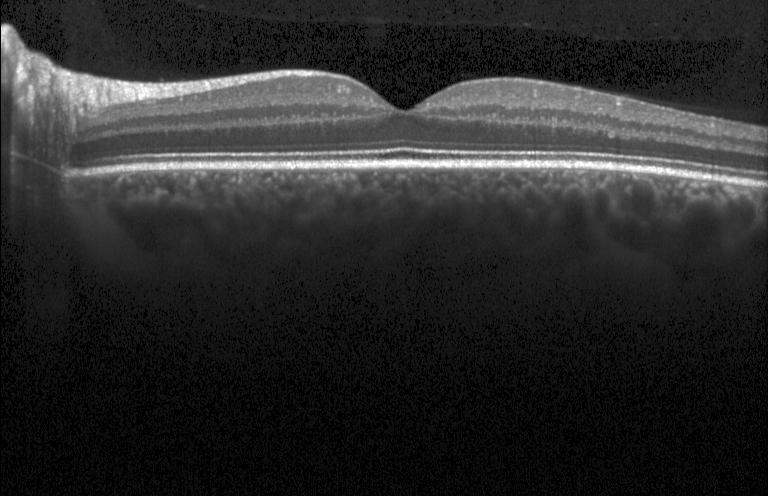 Acquired on a Heidelberg Spectralis, optical coherence tomography B-scan, centered on the fovea.
This B-scan demonstrates no choroidal neovascularization, no diabetic macular edema, and no drusen.